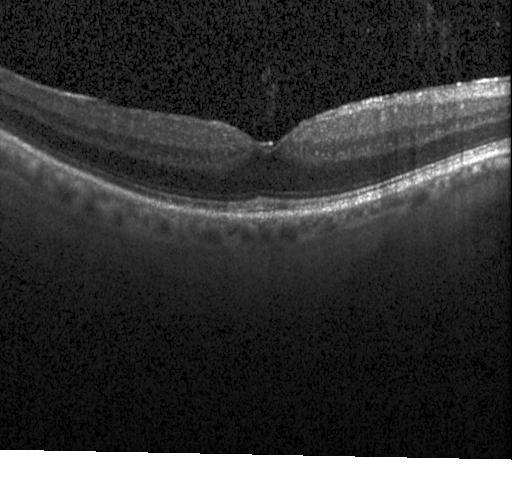

Macular OCT: no CNV, no DME, and no drusen.